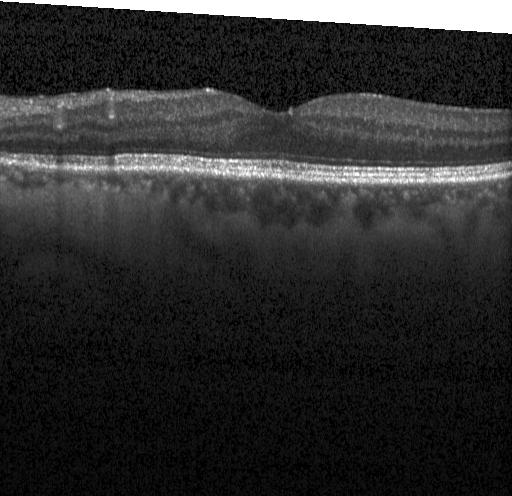 No evidence of choroidal neovascularization, diabetic macular edema, or drusen.